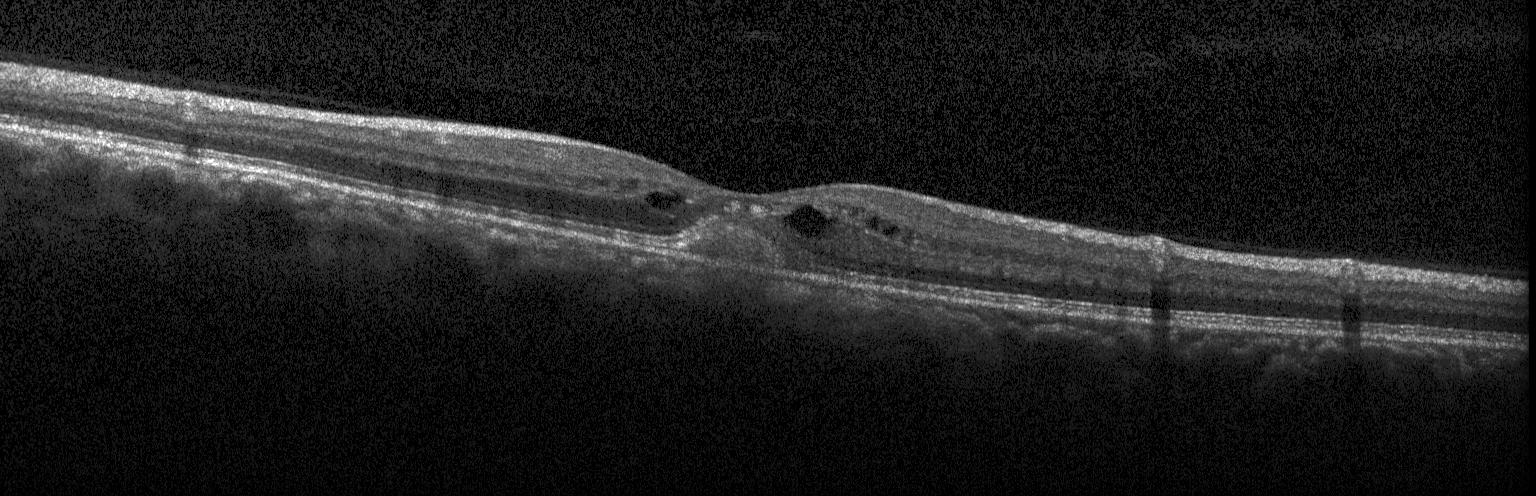

Retinal OCT B-scan — The scan shows a choroidal neovascular membrane.